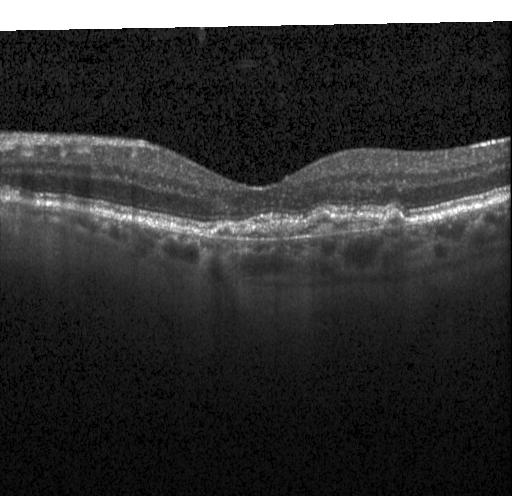
OCT finding: choroidal neovascularization (CNV).